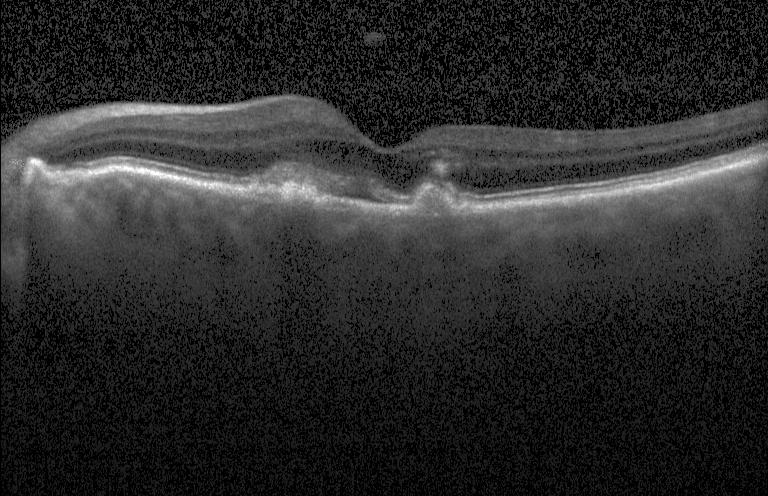

OCT B-scan; spectral-domain OCT
Finding: a choroidal neovascular membrane.